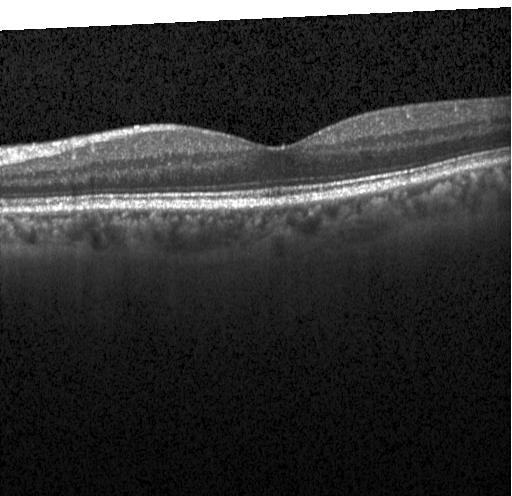 Impression: no choroidal neovascularization, no diabetic macular edema, and no drusen.